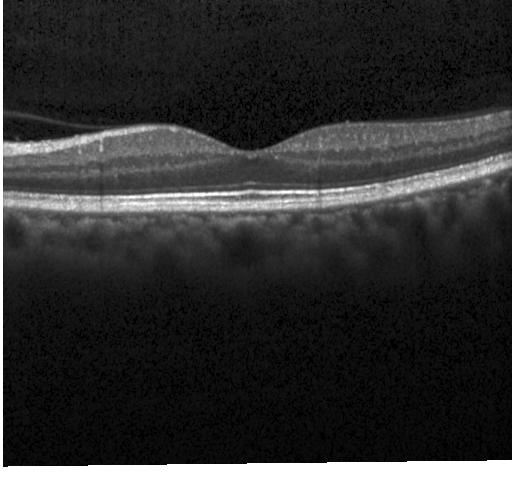
Optical coherence tomography scan — This B-scan demonstrates no choroidal neovascularization, diabetic macular edema, or drusen.